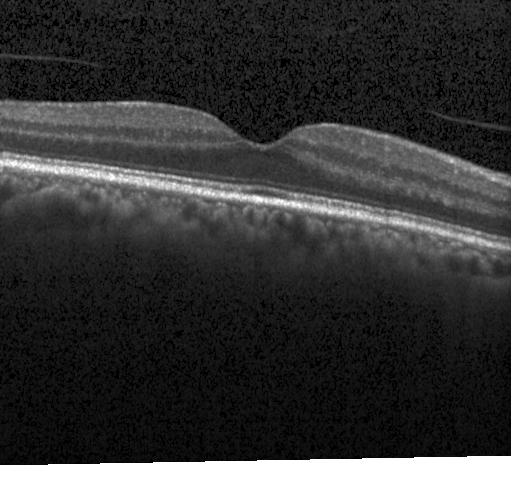 Finding: no CNV, no DME, and no drusen.